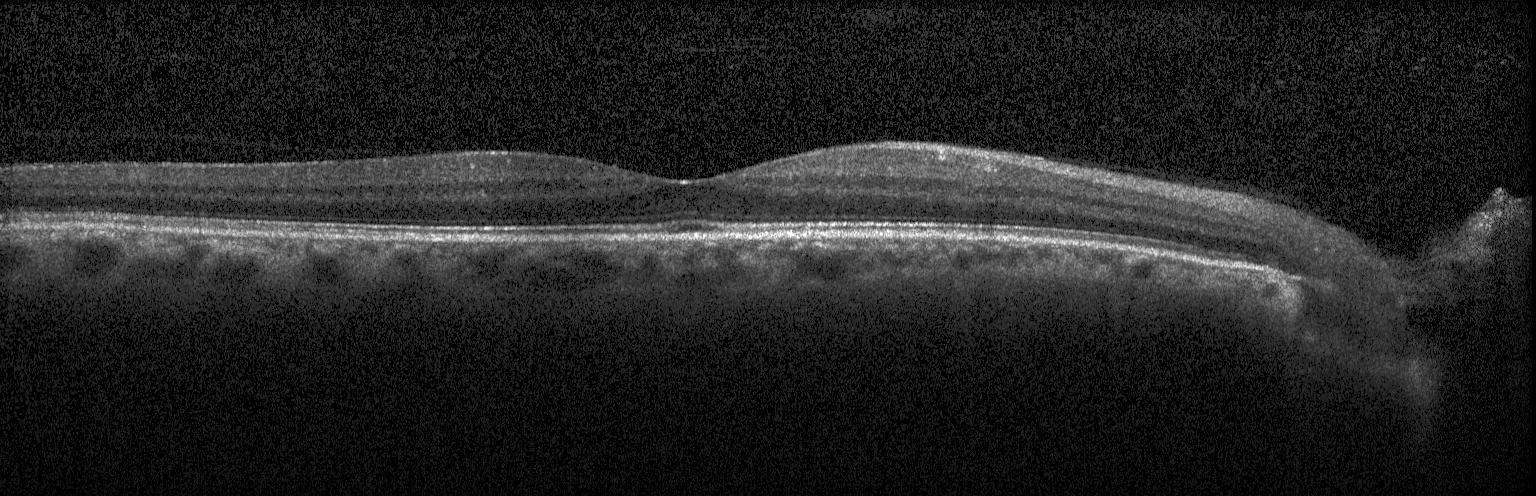

OCT B-scan showing no evidence of choroidal neovascularization, diabetic macular edema, or drusen.